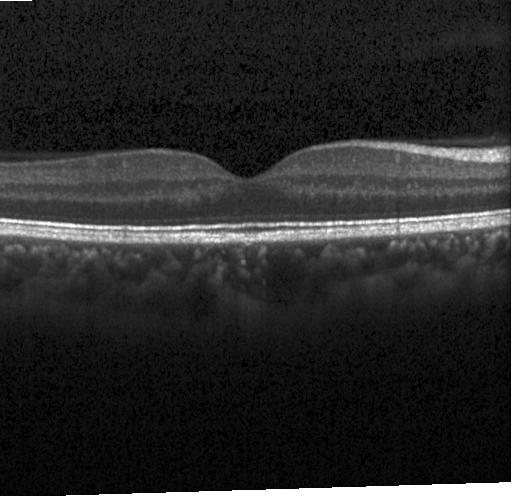

Optical coherence tomography B-scan. Macular scan
This B-scan demonstrates neither choroidal neovascularization, diabetic macular edema, nor drusen.